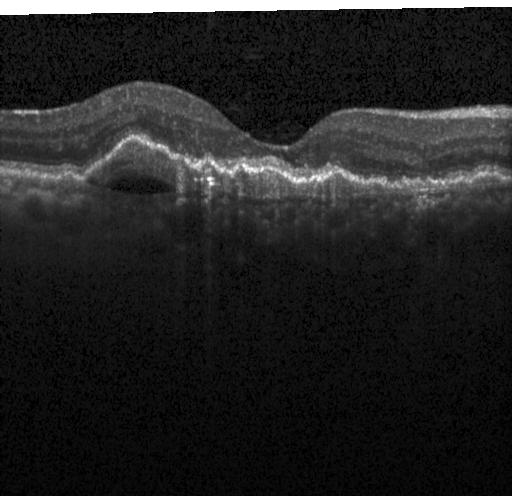
Diagnosis: choroidal neovascularization.